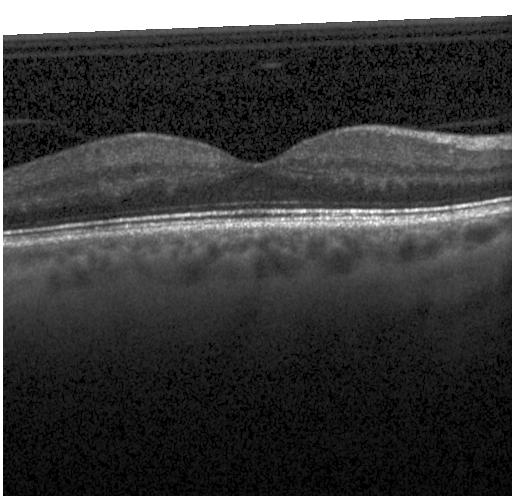 Heidelberg Spectralis, OCT line scan — Finding: neither choroidal neovascularization, diabetic macular edema, nor drusen.